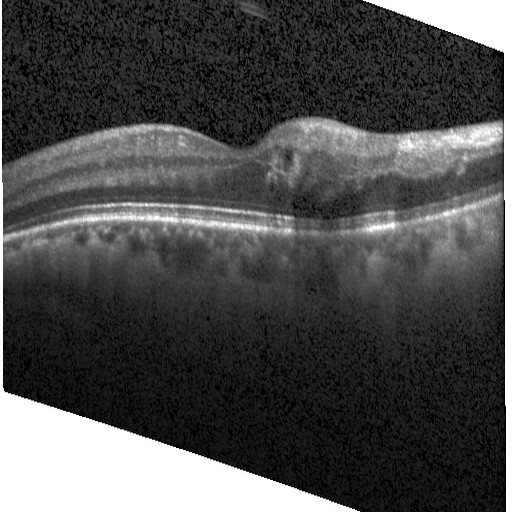 Through the macula; optical coherence tomography B-scan; SD-OCT. Impression: DME.